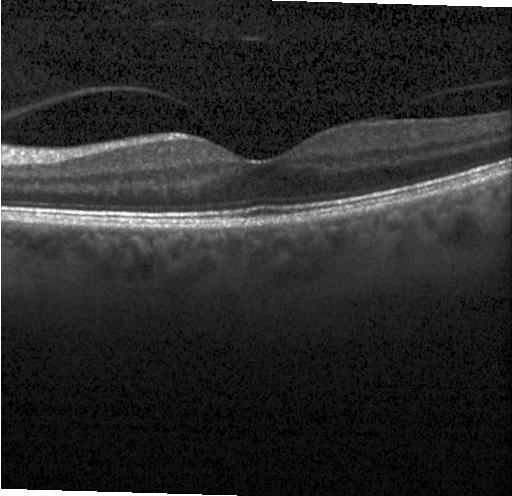

Spectral-domain OCT B-scan: no evidence of choroidal neovascularization, diabetic macular edema, or drusen.